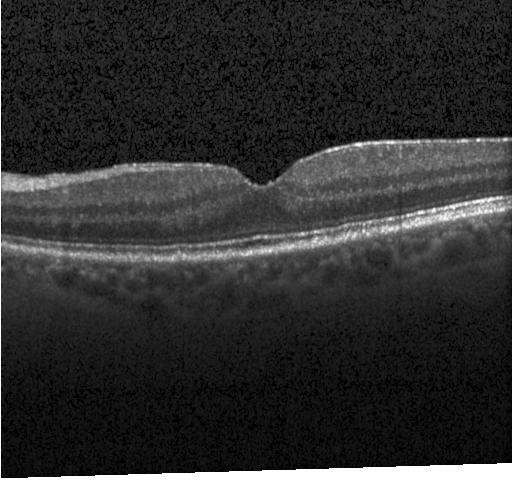
Optical coherence tomography B-scan — Finding: no evidence of choroidal neovascularization, diabetic macular edema, or drusen.